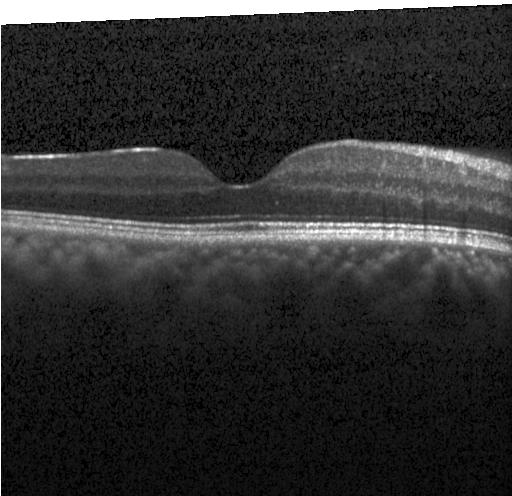

SD-OCT; fovea-centered; Heidelberg Spectralis OCT system; retinal OCT cross-section. Diagnosis: no CNV, no DME, and no drusen.